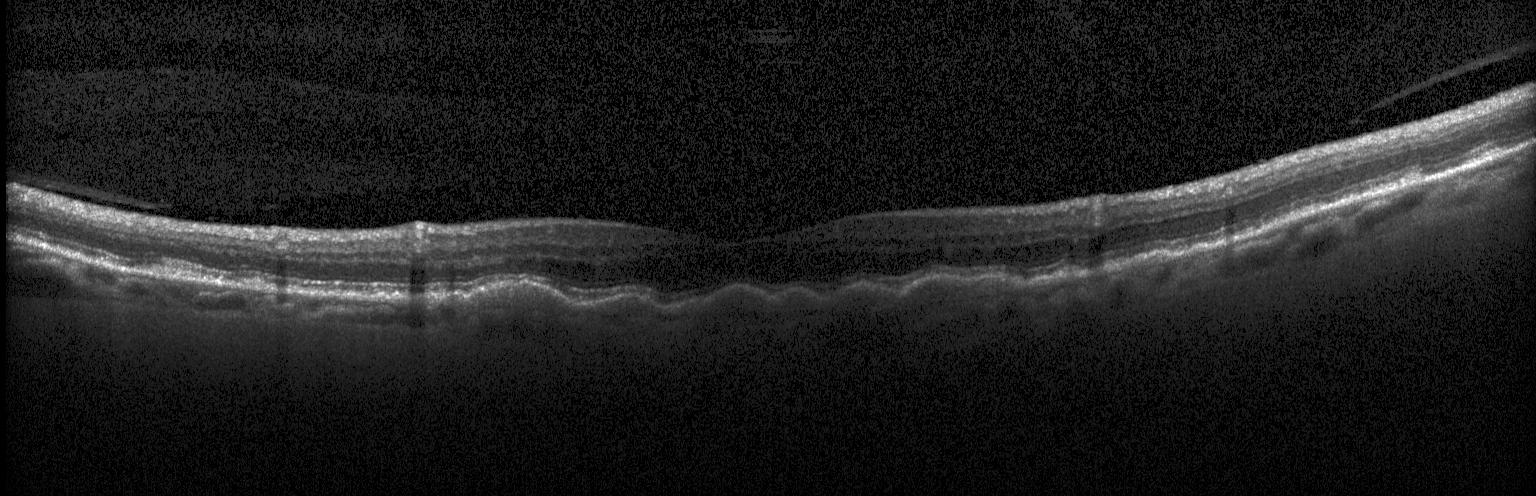
OCT finding: CNV.